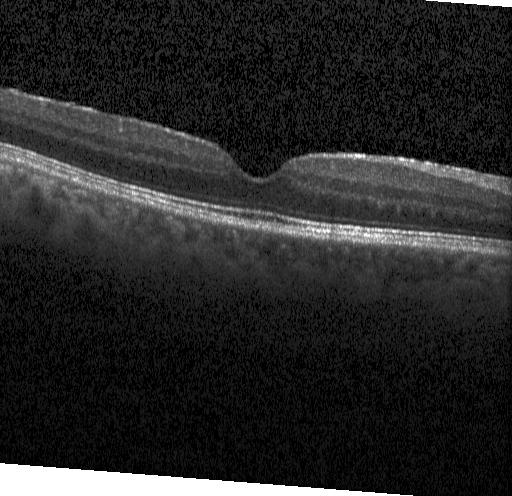

Acquired on a Heidelberg Spectralis, centered on the fovea, OCT line scan
The scan shows no CNV, DME, or drusen.